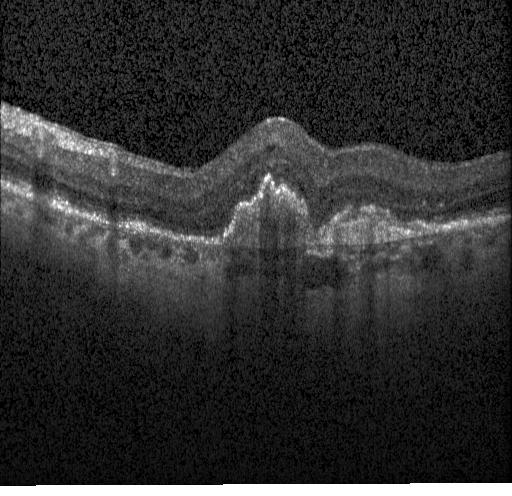 Impression: choroidal neovascularization (CNV).